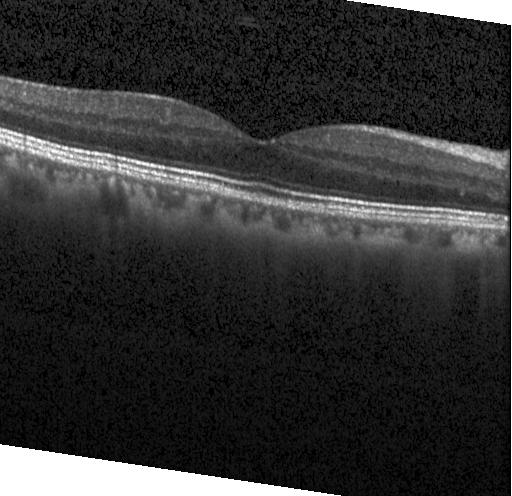 Retinal OCT B-scan.
Finding: no evidence of choroidal neovascularization, diabetic macular edema, or drusen.